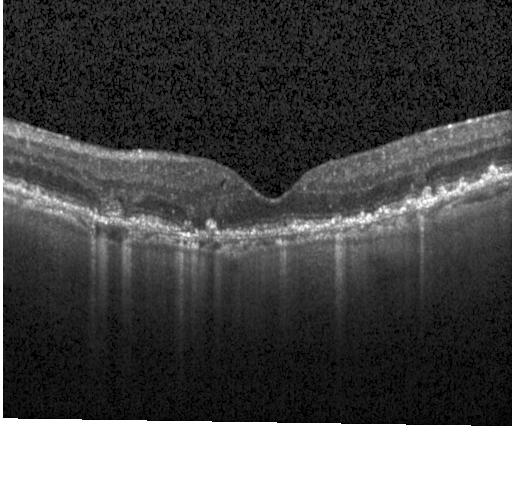 This B-scan demonstrates choroidal neovascularization (CNV).